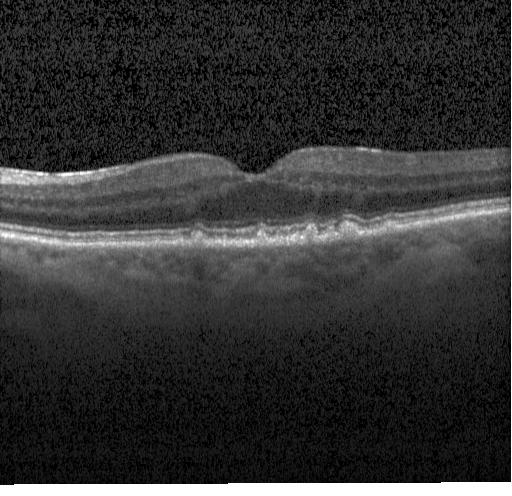

Retinal OCT cross-section. Through the macula. SD-OCT
Impression: sub-RPE drusenoid deposits.